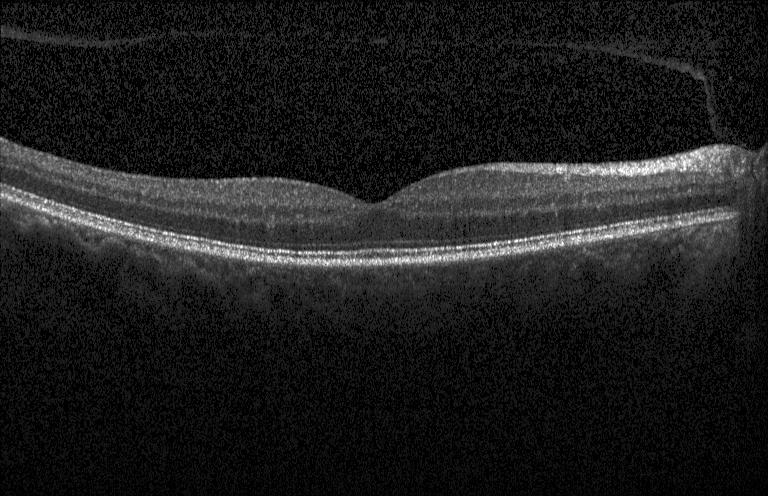

Spectral-domain optical coherence tomography · centered on the fovea · instrument: Heidelberg Spectralis · OCT B-scan.
Diagnosis: no CNV, DME, or drusen.